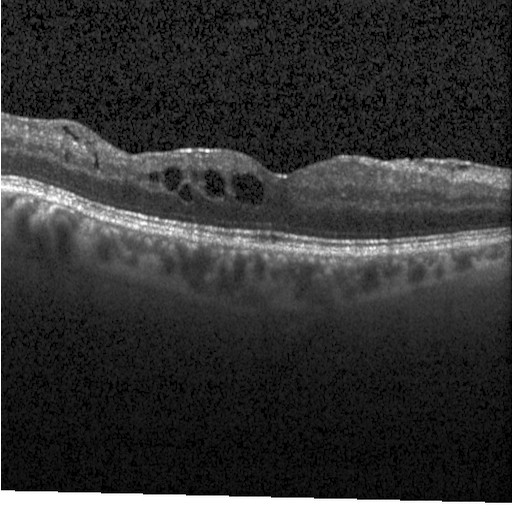

Diabetic macular edema.